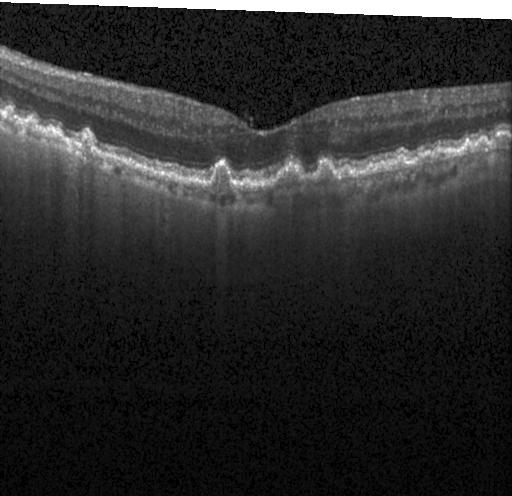

Centered on the fovea · OCT line scan — Impression: drusen.